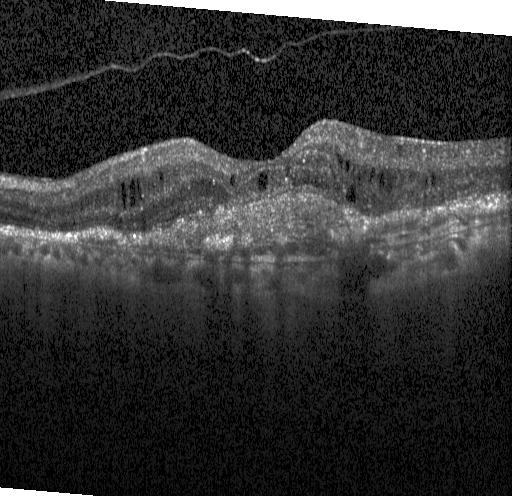
Retinal OCT cross-section — Finding: choroidal neovascularization (CNV).